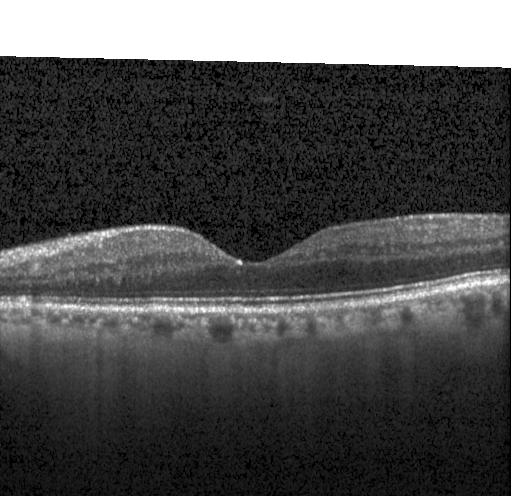 Finding: no CNV, DME, or drusen.